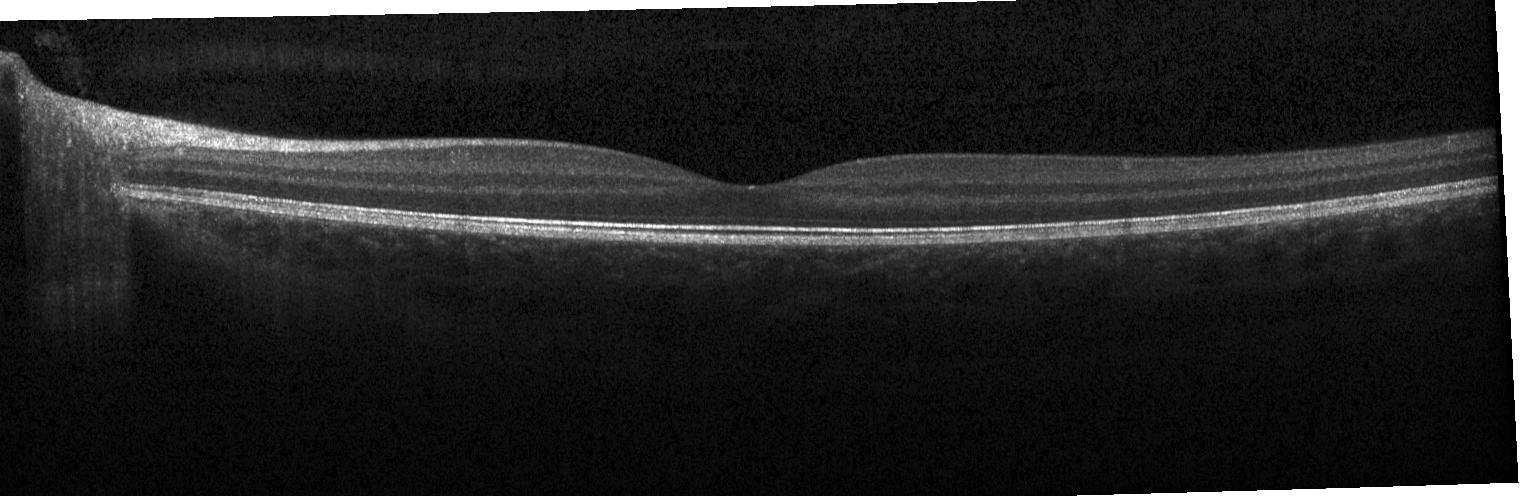 Through the macula; acquired on a Heidelberg Spectralis; SD-OCT; optical coherence tomography scan.
No choroidal neovascularization, no diabetic macular edema, and no drusen.